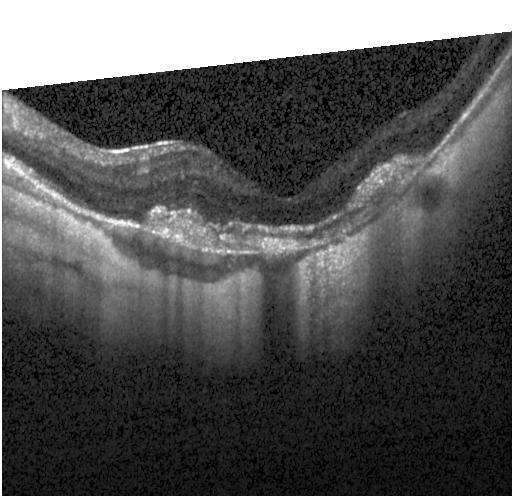 Macular OCT: CNV.